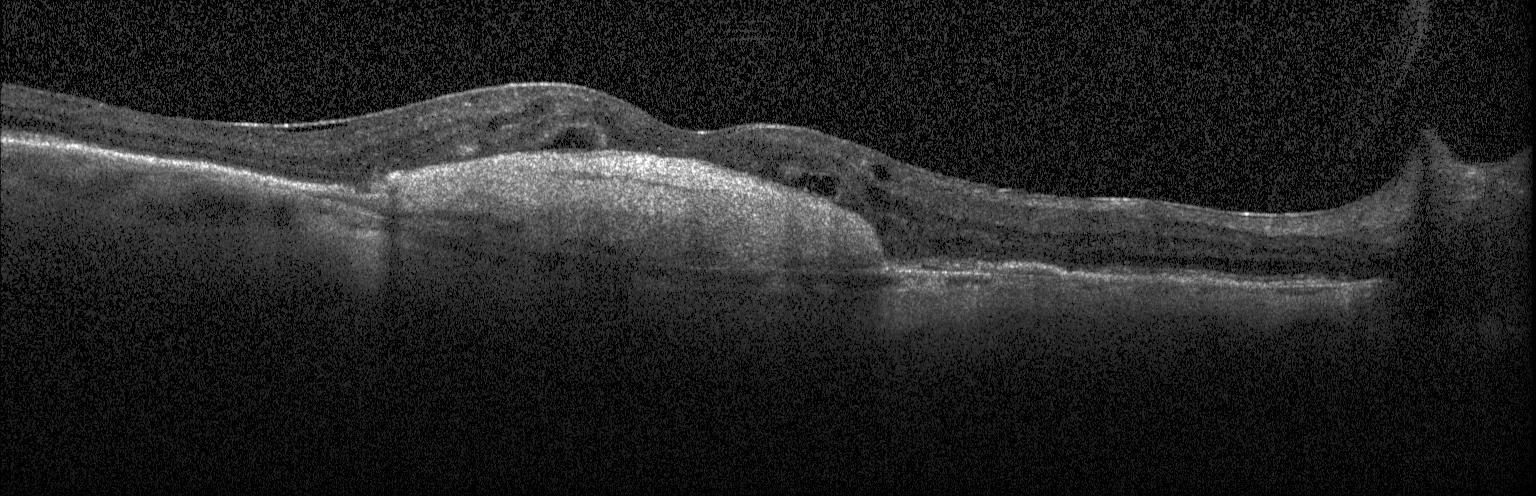
Macular OCT demonstrating choroidal neovascularization (CNV).